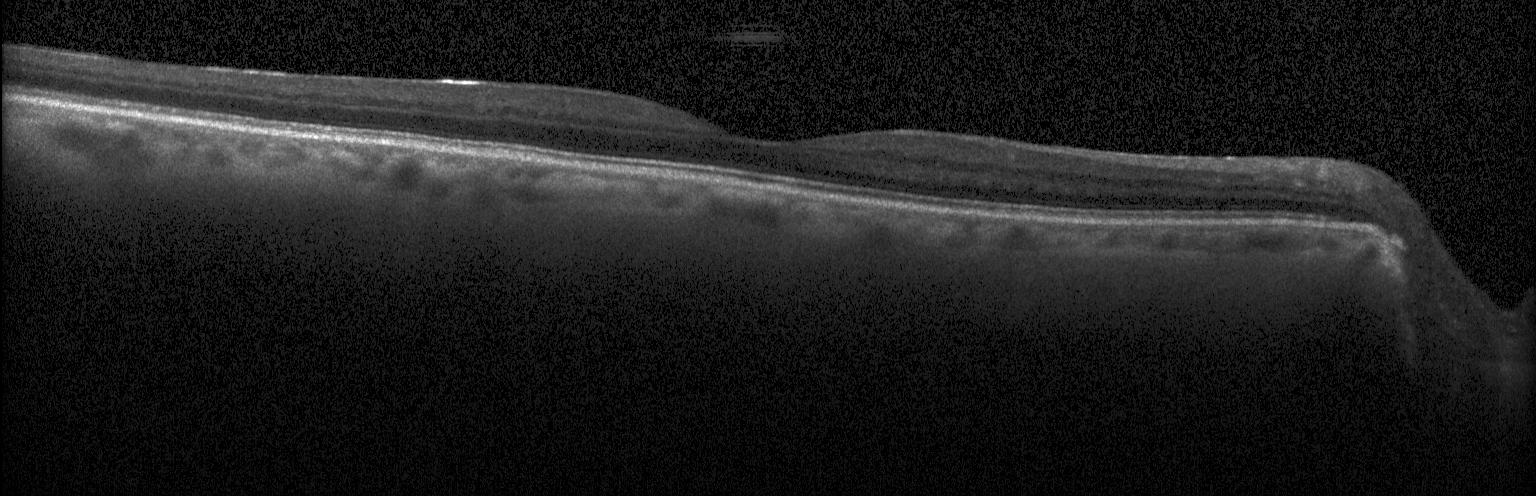

Retinal OCT cross-section · instrument: Heidelberg Spectralis · spectral-domain OCT. Impression: no CNV, DME, or drusen.